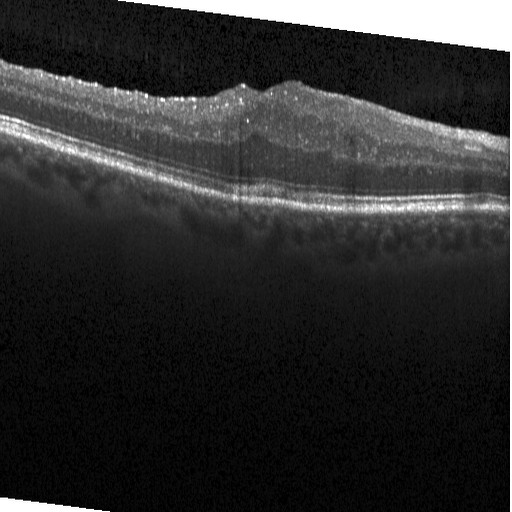
Diabetic macular edema (DME).